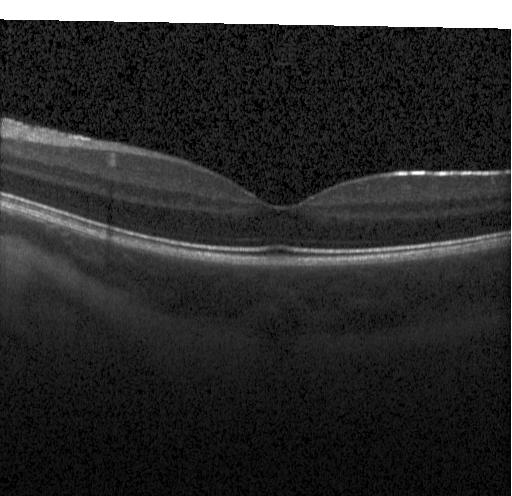

Optical coherence tomography scan; SD-OCT; instrument: Heidelberg Spectralis
Macular OCT: neither choroidal neovascularization, diabetic macular edema, nor drusen.